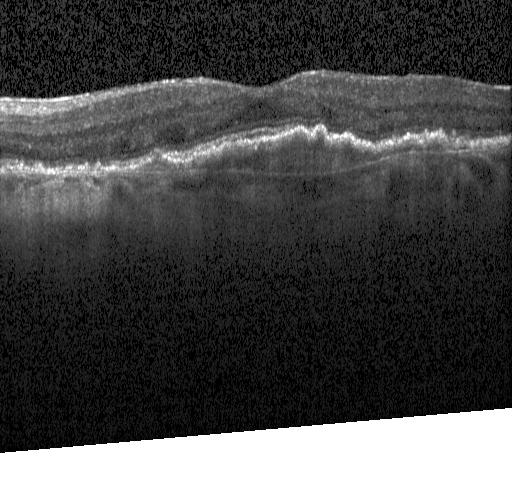 Macular OCT demonstrating choroidal neovascularization.